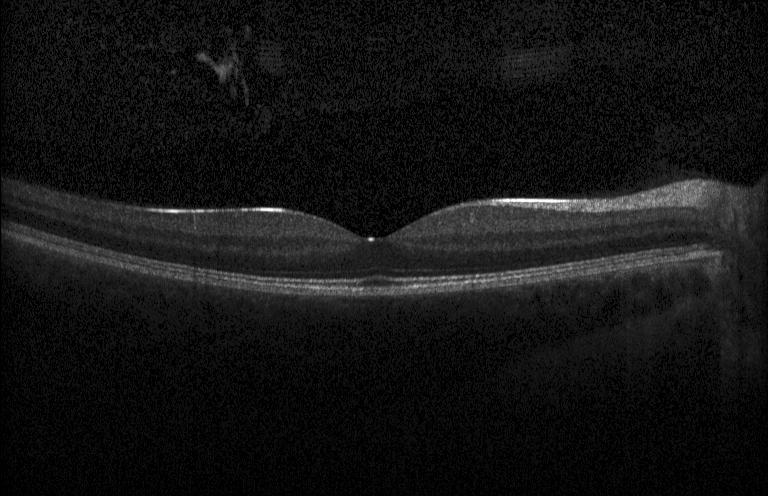

OCT B-scan.
Assessment: no evidence of CNV, DME, or drusen.